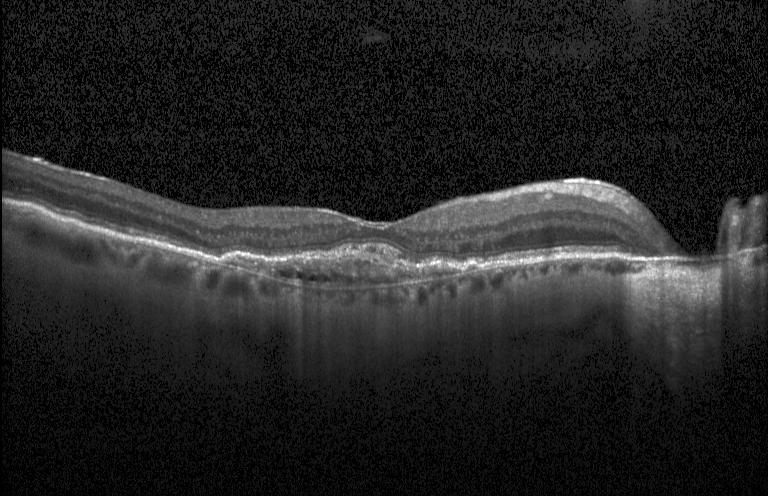
The scan shows a choroidal neovascular membrane.